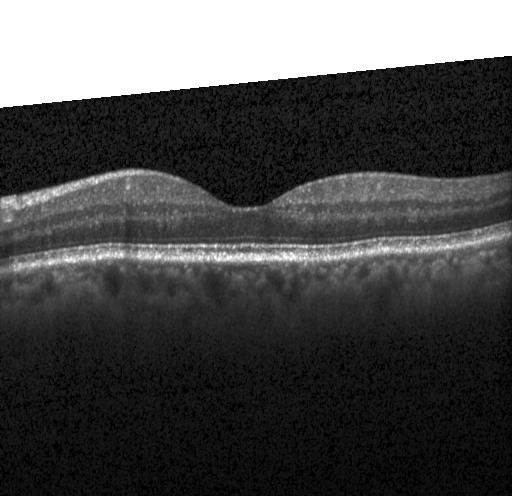
OCT line scan.
Impression: no evidence of CNV, DME, or drusen.